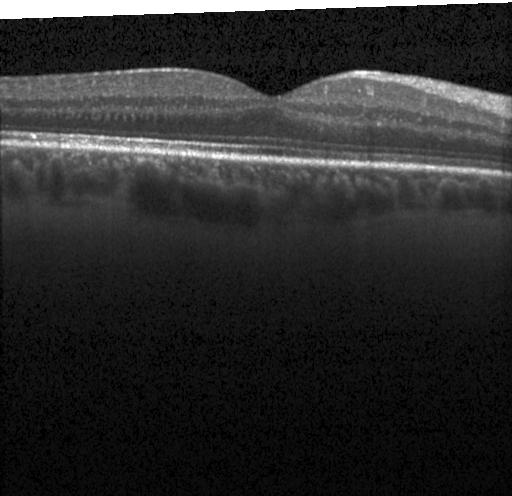 OCT scan showing no CNV, no DME, and no drusen.